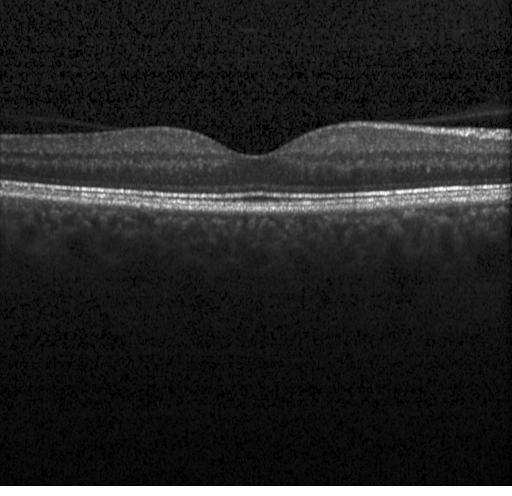 Retinal OCT B-scan — Impression: no CNV, no DME, and no drusen.